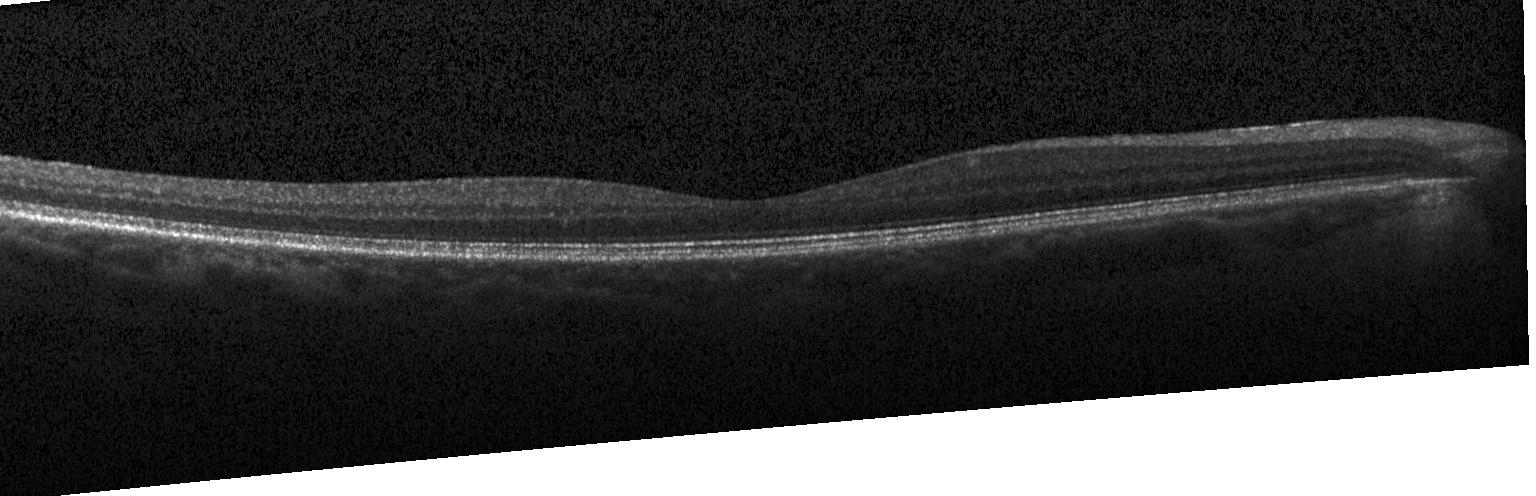

OCT finding: no evidence of choroidal neovascularization, diabetic macular edema, or drusen.